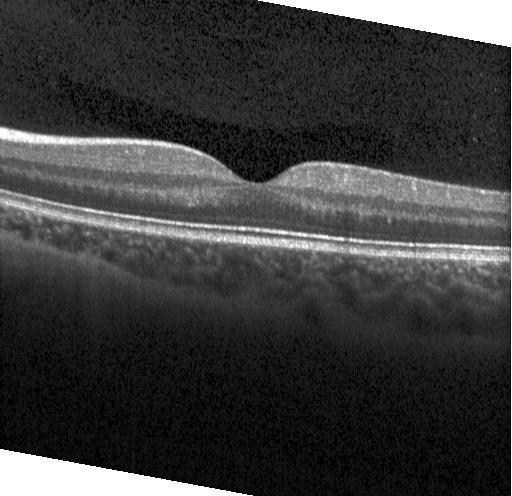 Finding: no evidence of choroidal neovascularization, diabetic macular edema, or drusen.